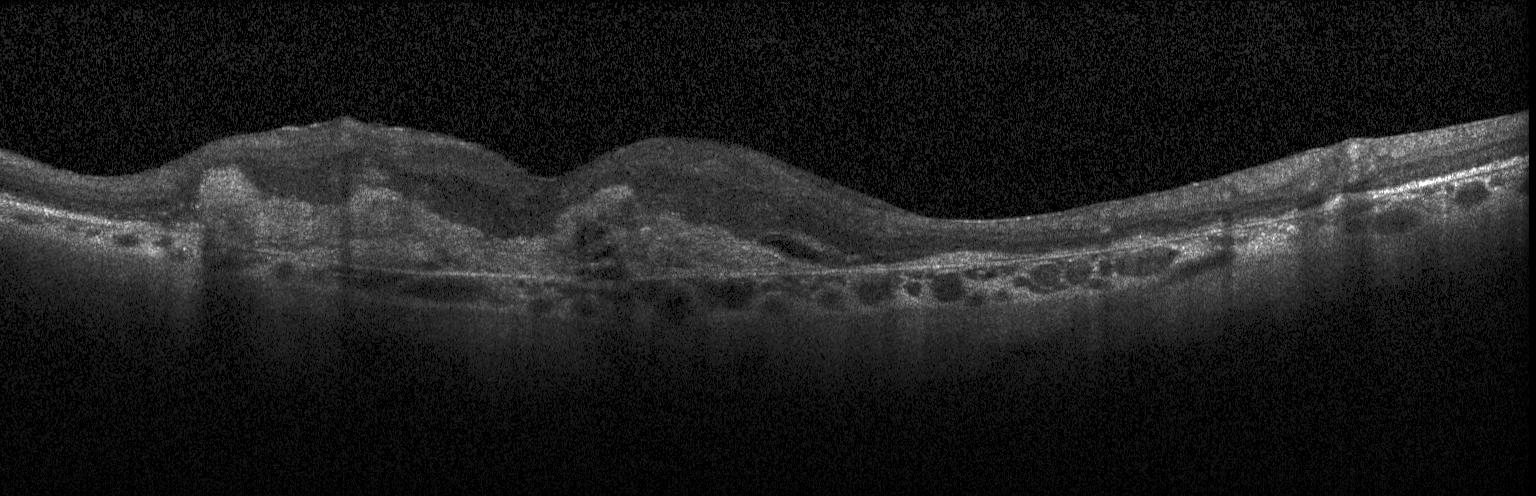
Diagnosis: a choroidal neovascular membrane.